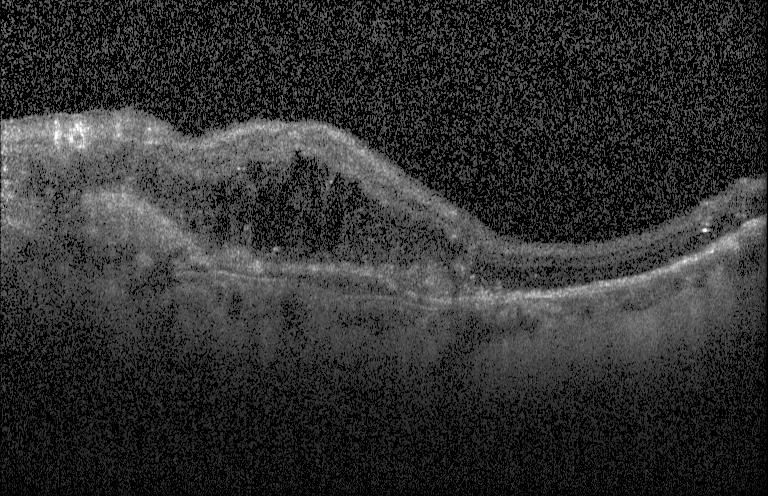 This B-scan demonstrates choroidal neovascularization.